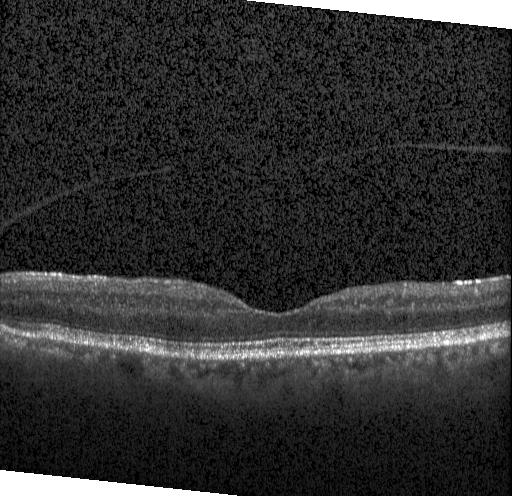 SD-OCT · retinal OCT B-scan.
Assessment: no CNV, no DME, and no drusen.